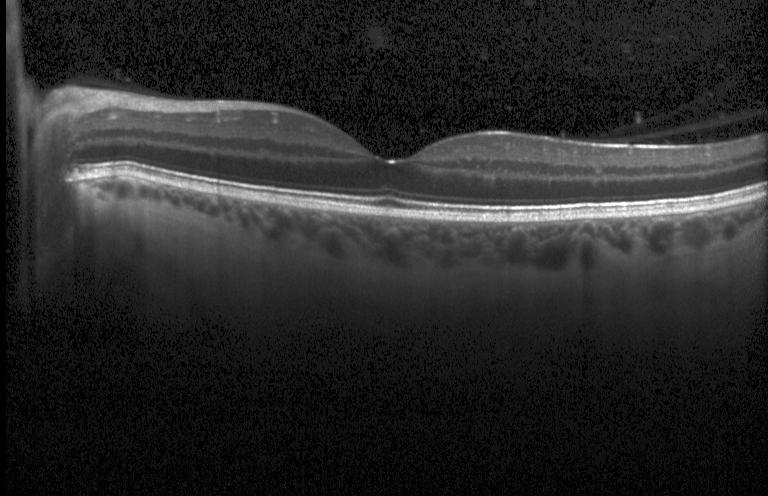 OCT B-scan.
Macular OCT: no choroidal neovascularization, no diabetic macular edema, and no drusen.